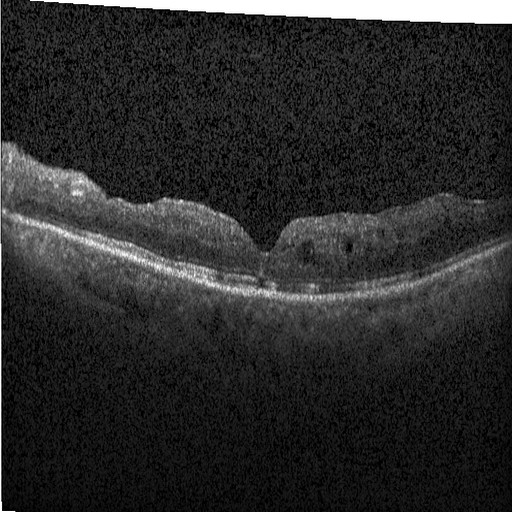
Macular OCT demonstrating diabetic macular edema.